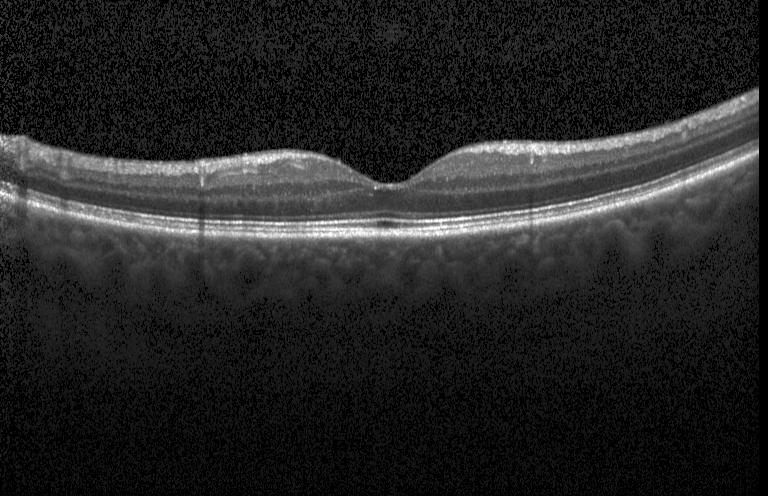 Macular OCT: no evidence of choroidal neovascularization, diabetic macular edema, or drusen.